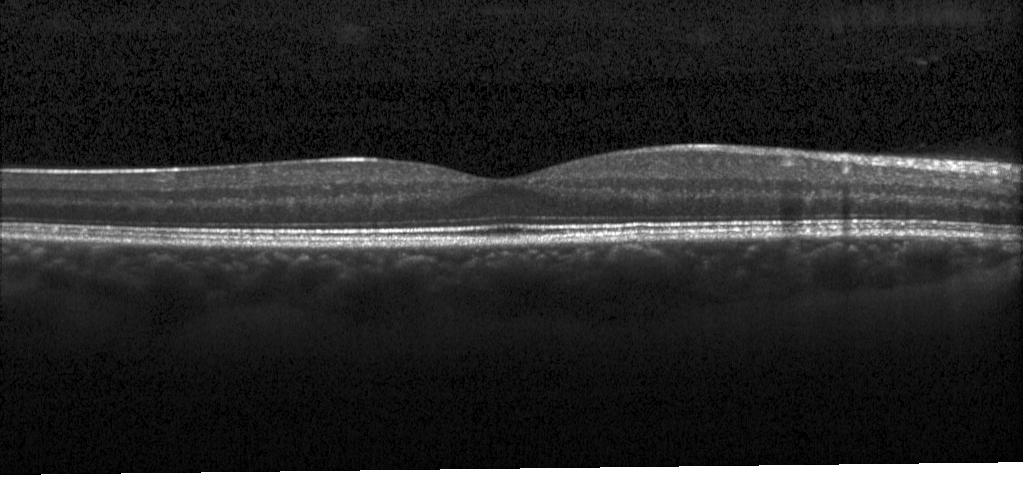 OCT B-scan showing no choroidal neovascularization, diabetic macular edema, or drusen.